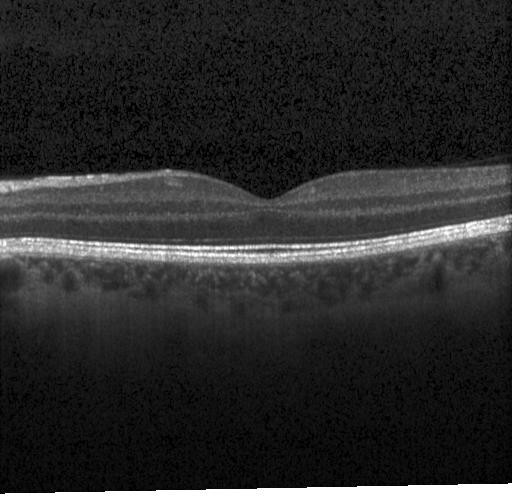
OCT finding: neither choroidal neovascularization, diabetic macular edema, nor drusen.